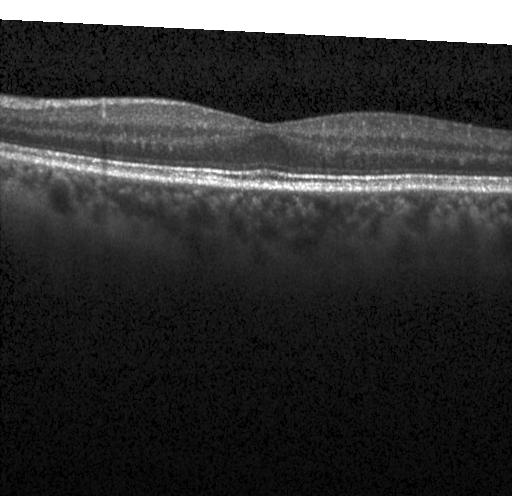

OCT line scan.
OCT finding: no evidence of choroidal neovascularization, diabetic macular edema, or drusen.